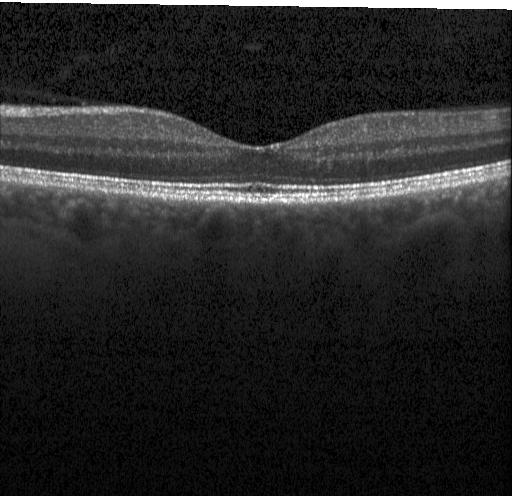
Fovea-centered, SD-OCT, optical coherence tomography B-scan
Impression: neither choroidal neovascularization, diabetic macular edema, nor drusen.